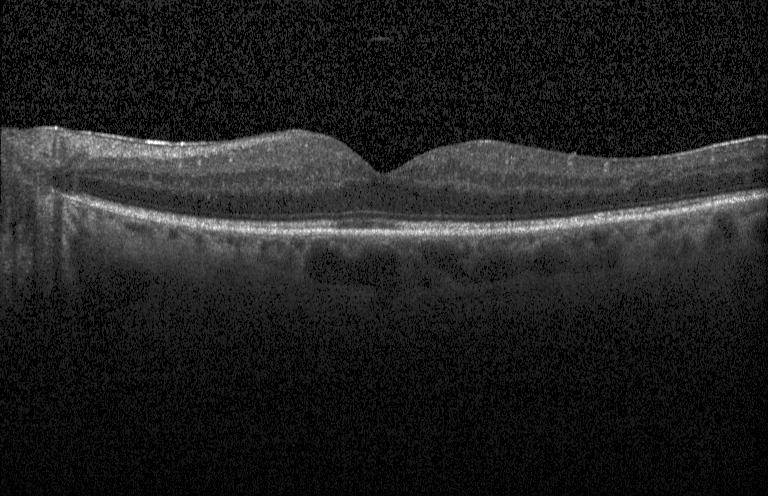 Optical coherence tomography scan
Impression: neither choroidal neovascularization, diabetic macular edema, nor drusen.